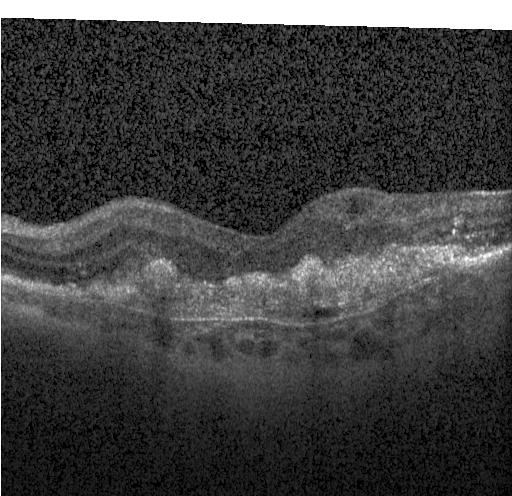

Macular scan · instrument: Heidelberg Spectralis · SD-OCT · retinal OCT B-scan — OCT finding: choroidal neovascularization (CNV).